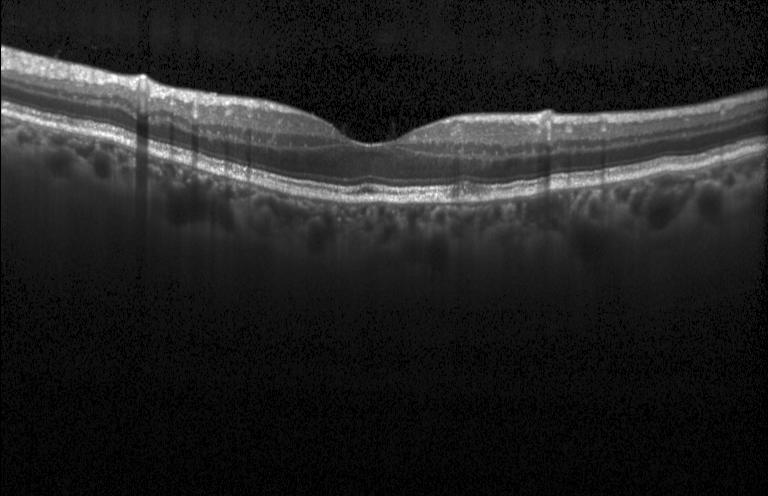
OCT scan showing no CNV, no DME, and no drusen.